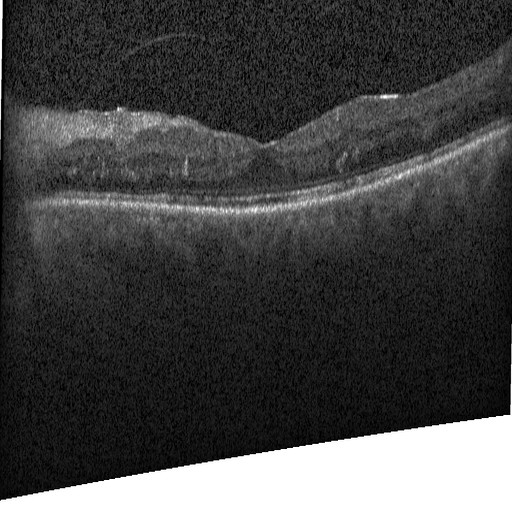
Finding: diabetic macular edema.